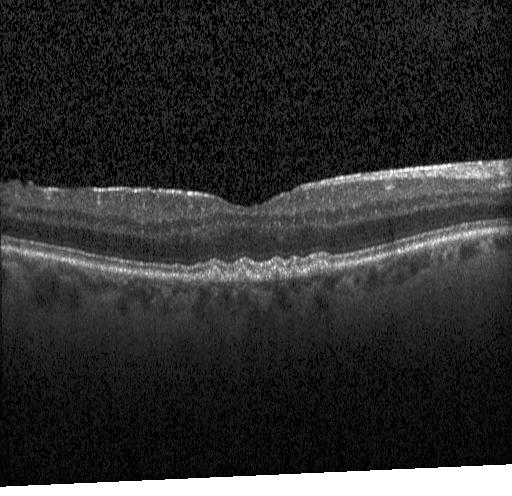 Optical coherence tomography scan
Finding: drusen.